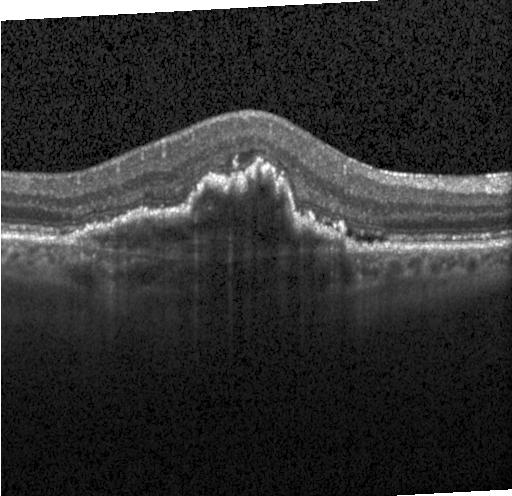 OCT B-scan showing CNV.